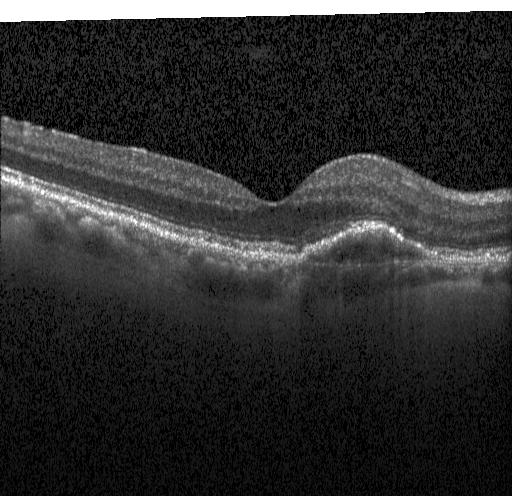

Impression: a choroidal neovascular membrane.